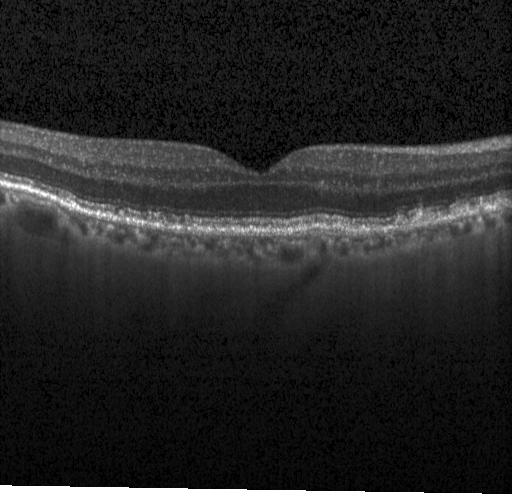 OCT B-scan.
Diagnosis: sub-RPE drusenoid deposits.